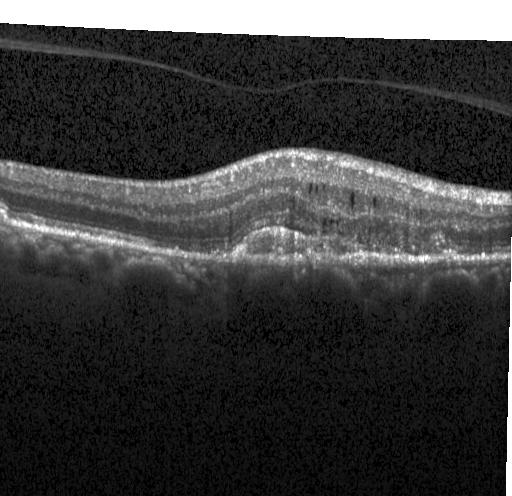

Retinal OCT cross-section; through the macula; Heidelberg Spectralis OCT system; spectral-domain optical coherence tomography
Impression: CNV.